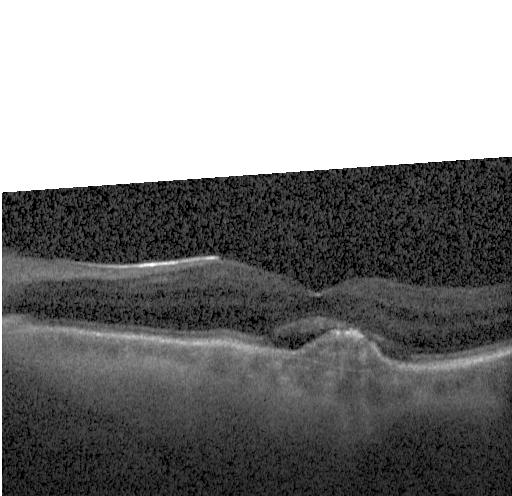
Retinal OCT B-scan.
Macular OCT: a choroidal neovascular membrane.